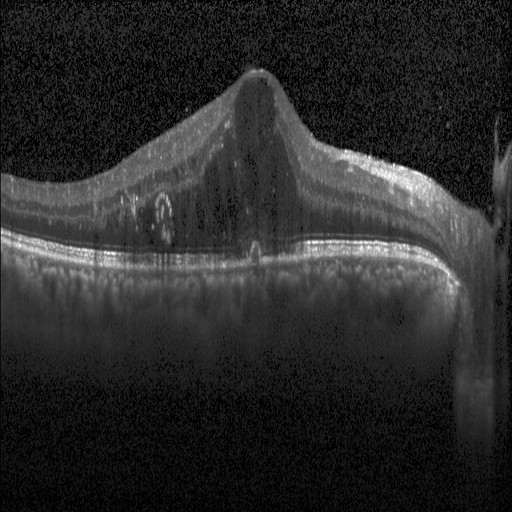

Spectral-domain OCT; fovea-centered; Heidelberg Spectralis OCT system; optical coherence tomography B-scan.
Diagnosis: DME.